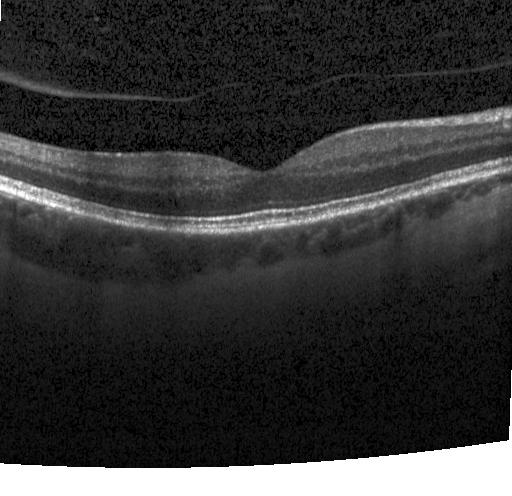 Impression: no CNV, no DME, and no drusen.